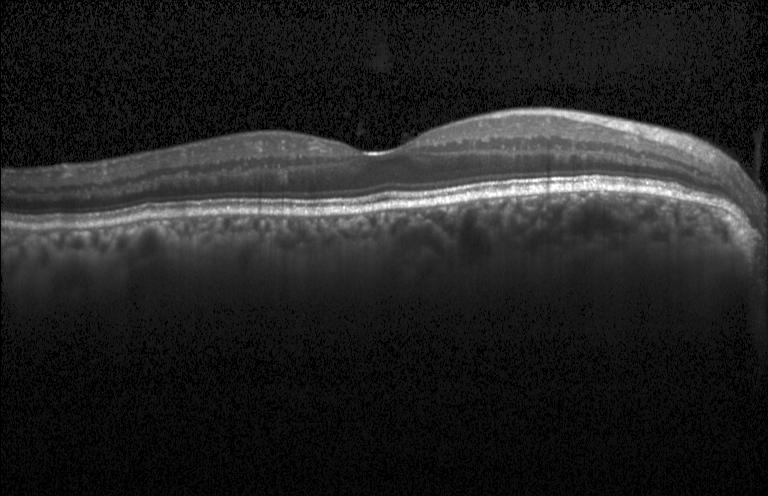
Heidelberg Spectralis. Through the macula. Retinal OCT cross-section. Spectral-domain OCT. Dx: no evidence of choroidal neovascularization, diabetic macular edema, or drusen.